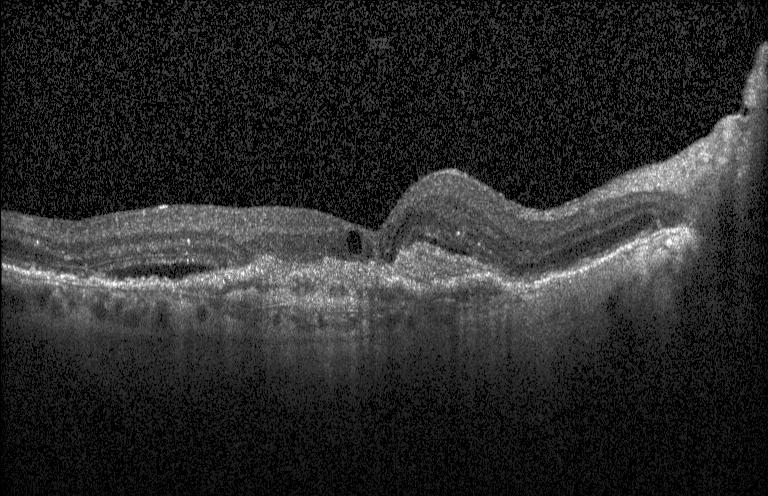 Optical coherence tomography B-scan — Diagnosis: a choroidal neovascular membrane.